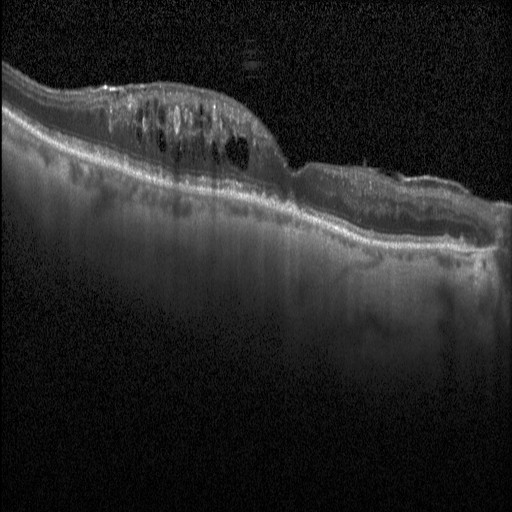
Retinal OCT B-scan. Heidelberg Spectralis OCT system. Through the macula
Impression: diabetic macular edema.